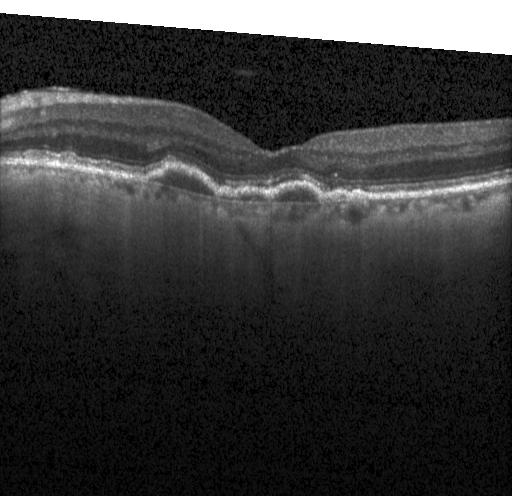 Heidelberg Spectralis, spectral-domain OCT, OCT line scan — A choroidal neovascular membrane.